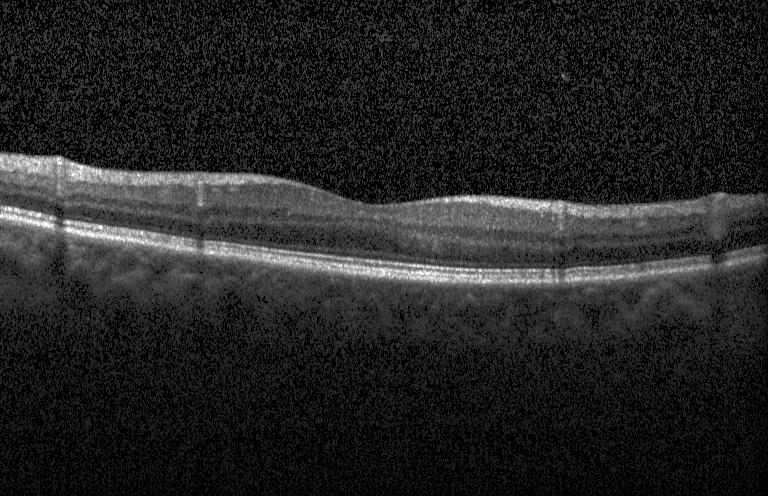

Optical coherence tomography scan. Neither choroidal neovascularization, diabetic macular edema, nor drusen.